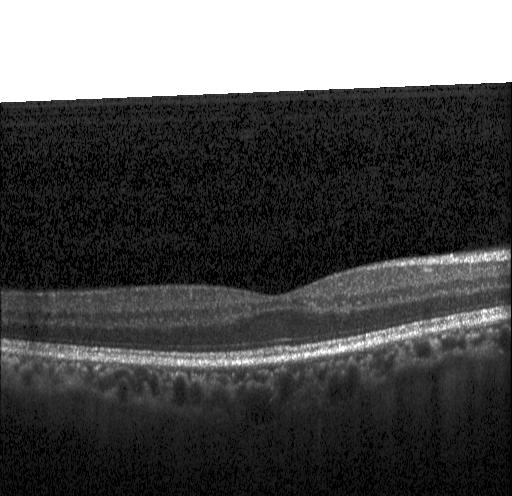 Spectral-domain OCT. OCT line scan
Dx: no choroidal neovascularization, diabetic macular edema, or drusen.